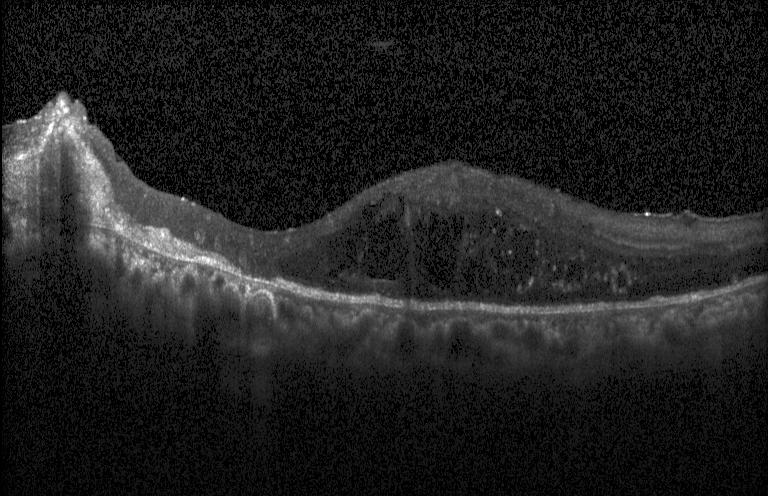
OCT B-scan; SD-OCT
This B-scan demonstrates a choroidal neovascular membrane.